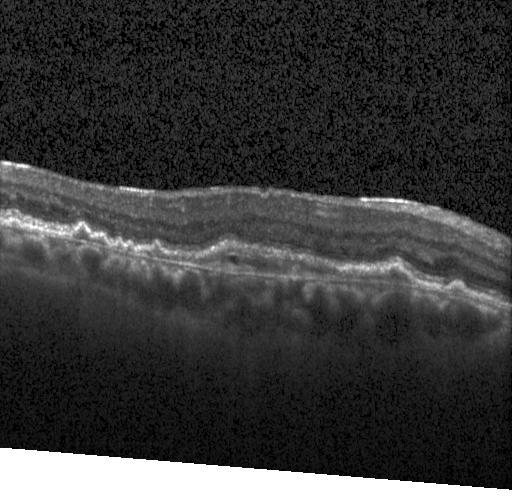

Finding: a choroidal neovascular membrane.